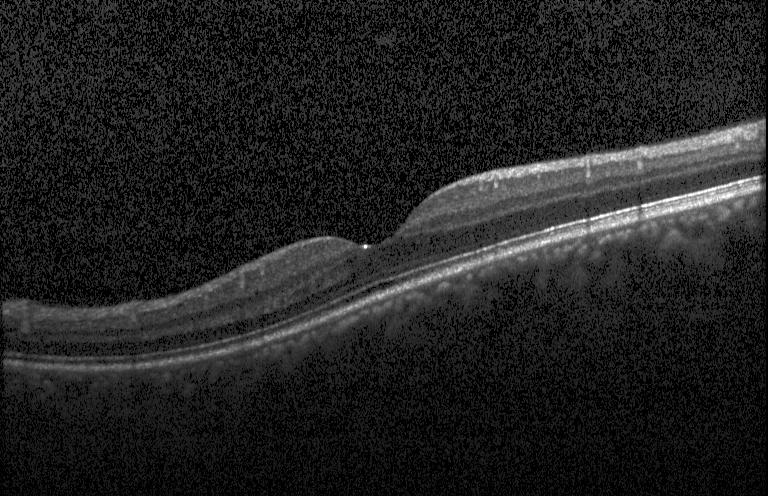 Macular OCT demonstrating no evidence of CNV, DME, or drusen.